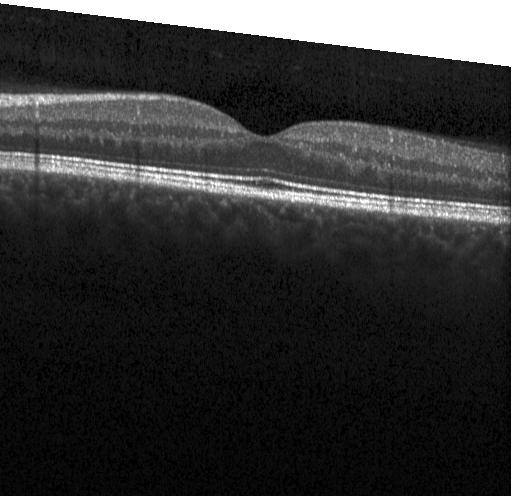

Macular scan, optical coherence tomography B-scan, spectral-domain optical coherence tomography
Impression: no CNV, DME, or drusen.